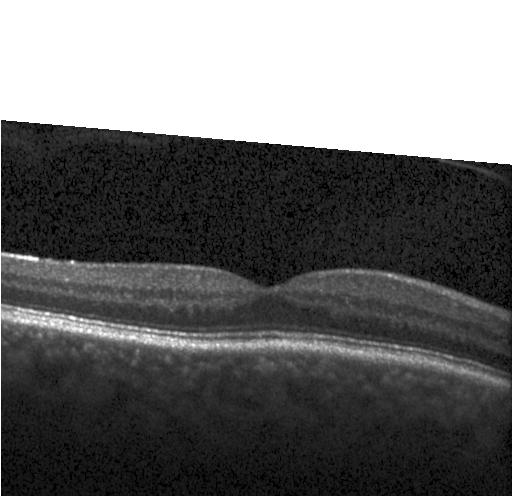
Retinal OCT B-scan, spectral-domain OCT, acquired on a Heidelberg Spectralis
Diagnosis: no choroidal neovascularization, diabetic macular edema, or drusen.